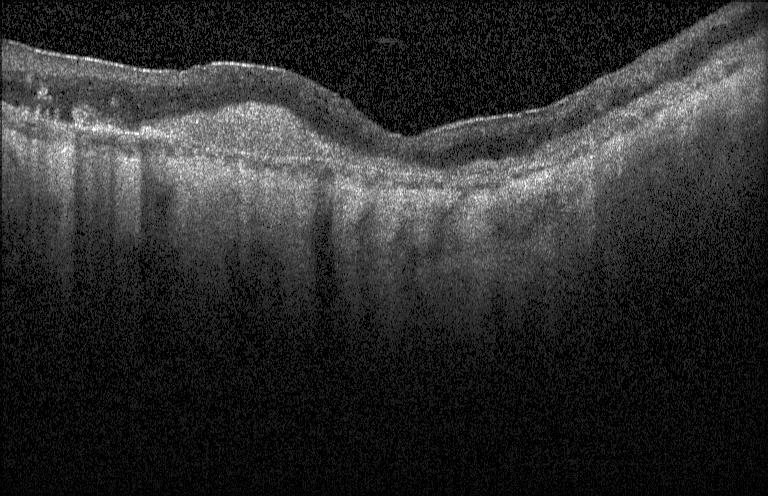 SD-OCT. Acquired on a Heidelberg Spectralis. Fovea-centered. Retinal OCT B-scan — Finding: a choroidal neovascular membrane.